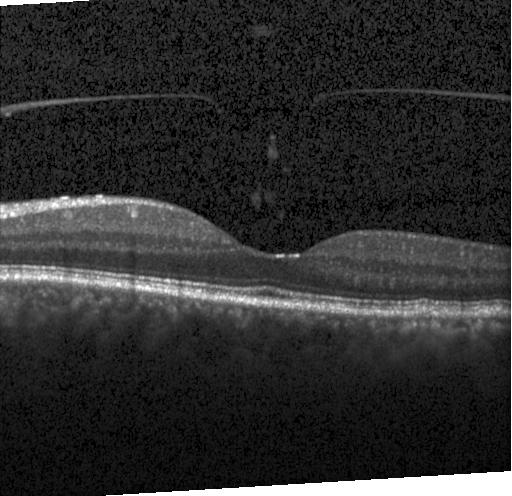
Spectral-domain optical coherence tomography, centered on the fovea, Heidelberg Spectralis, optical coherence tomography scan — The scan shows neither CNV, DME, nor drusen.